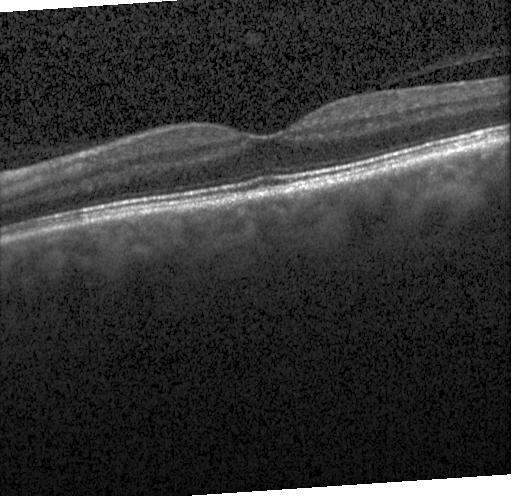 Horizontal scan through the fovea, retinal OCT B-scan. The scan shows no CNV, no DME, and no drusen.